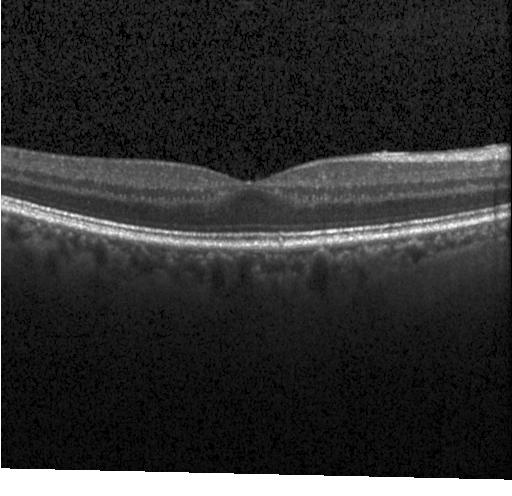
Through the macula. Heidelberg Spectralis OCT system. Retinal OCT B-scan — The scan shows no evidence of choroidal neovascularization, diabetic macular edema, or drusen.